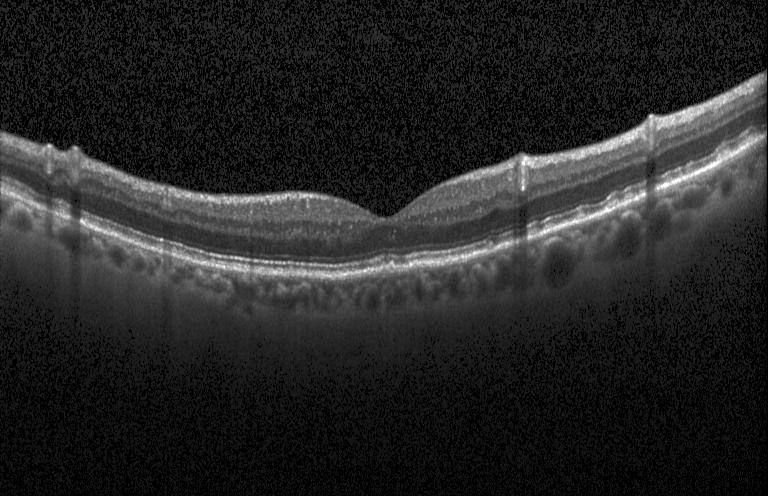
Heidelberg Spectralis. Retinal OCT B-scan. Fovea-centered — This B-scan demonstrates no CNV, no DME, and no drusen.